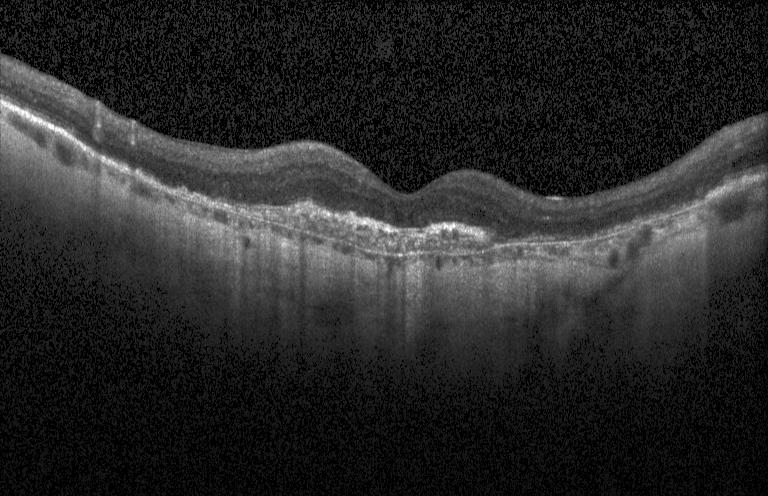

Macular OCT: a choroidal neovascular membrane.